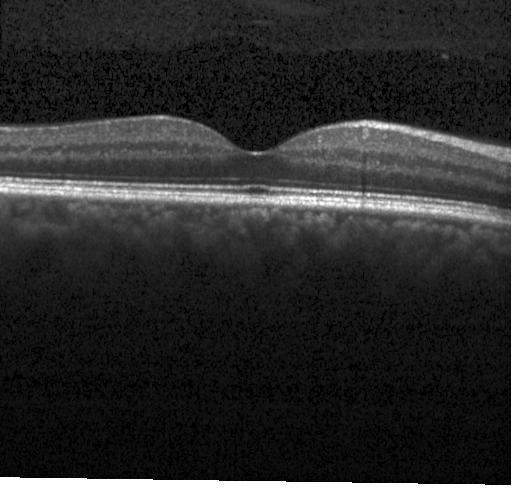 Diagnosis: no choroidal neovascularization, diabetic macular edema, or drusen.